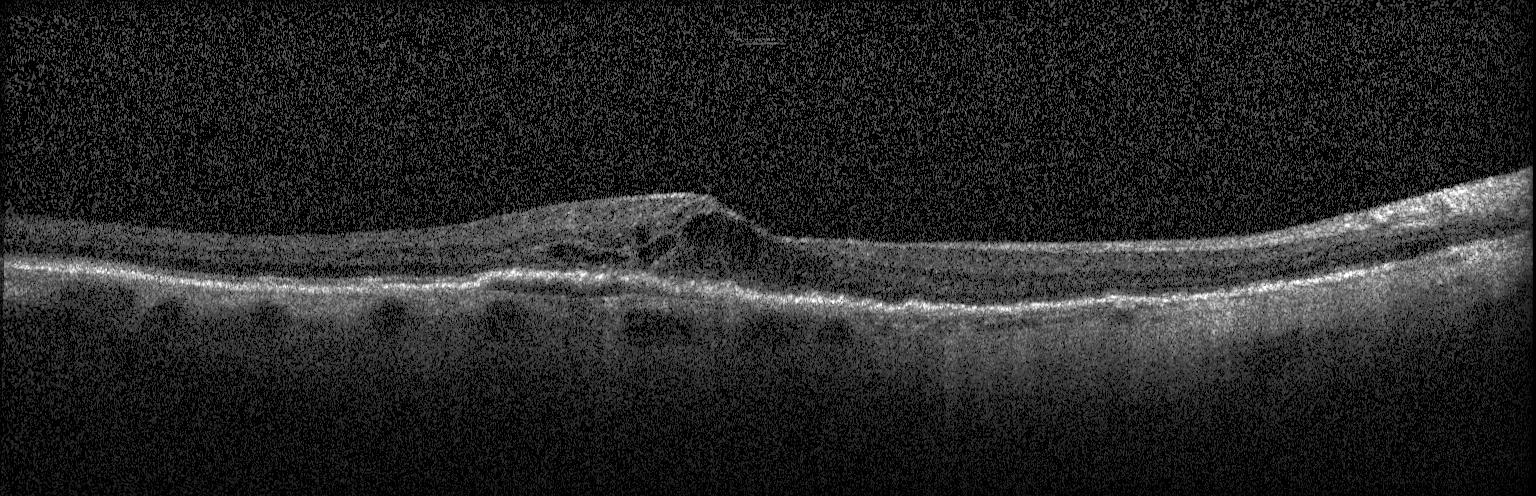

Assessment: a choroidal neovascular membrane.